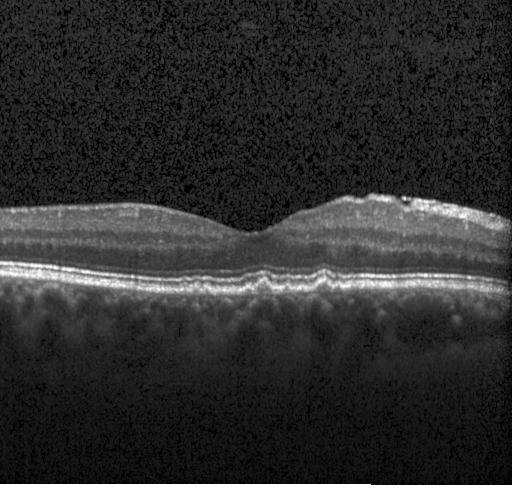 Macular scan · instrument: Heidelberg Spectralis · optical coherence tomography B-scan · SD-OCT
Finding: sub-RPE drusenoid deposits.